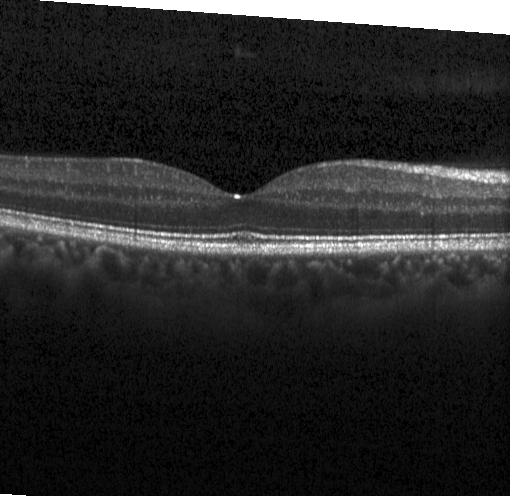 Optical coherence tomography scan, centered on the fovea, spectral-domain optical coherence tomography, instrument: Heidelberg Spectralis — The scan shows no choroidal neovascularization, diabetic macular edema, or drusen.